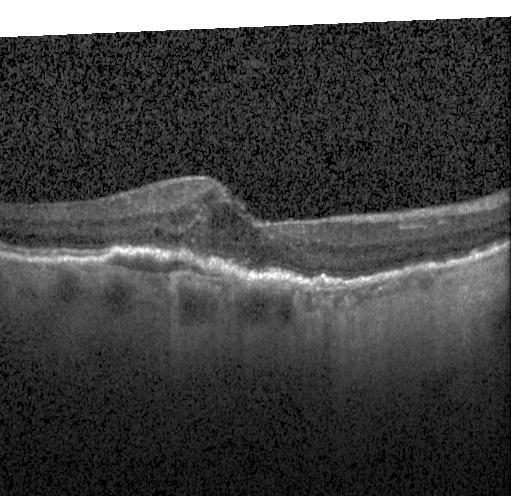
Retinal OCT B-scan.
This B-scan demonstrates CNV.